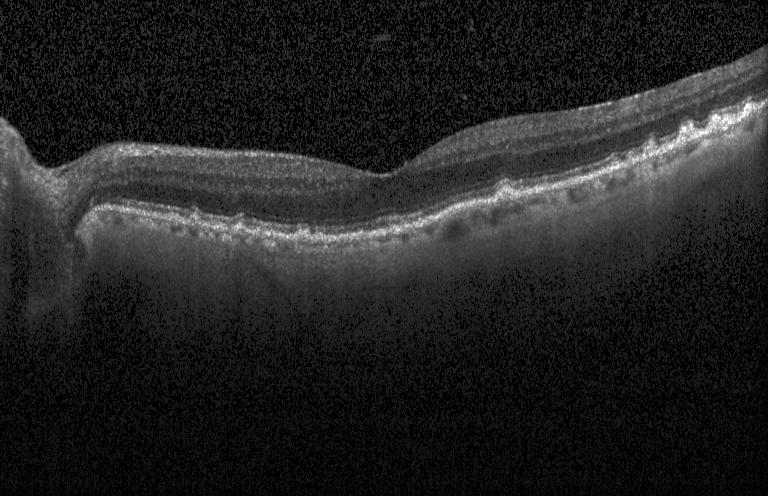
Heidelberg Spectralis; OCT line scan.
Impression: multiple drusen.